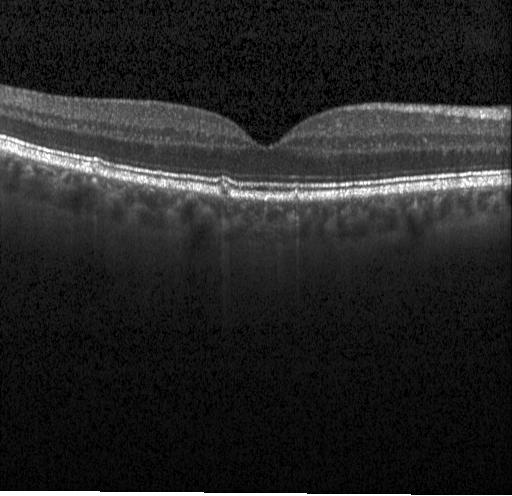

OCT scan showing multiple drusen.